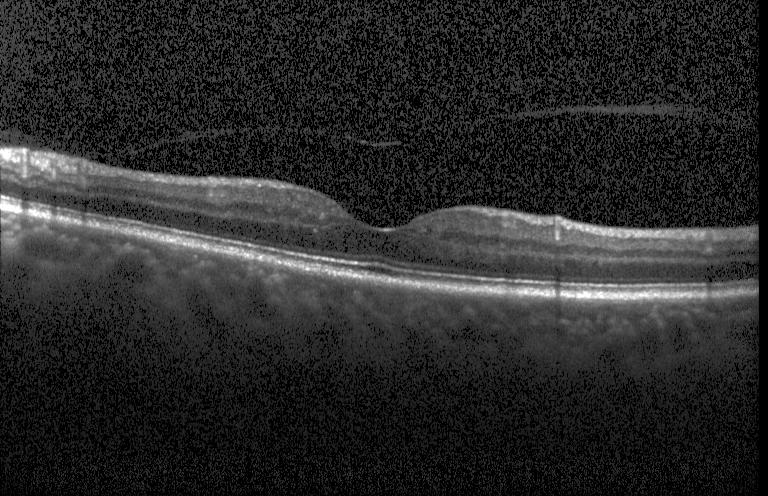

Retinal OCT B-scan.
Dx: no CNV, DME, or drusen.